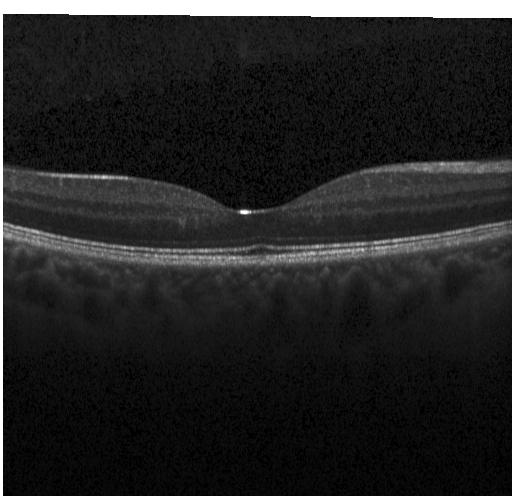
Finding: no evidence of CNV, DME, or drusen.